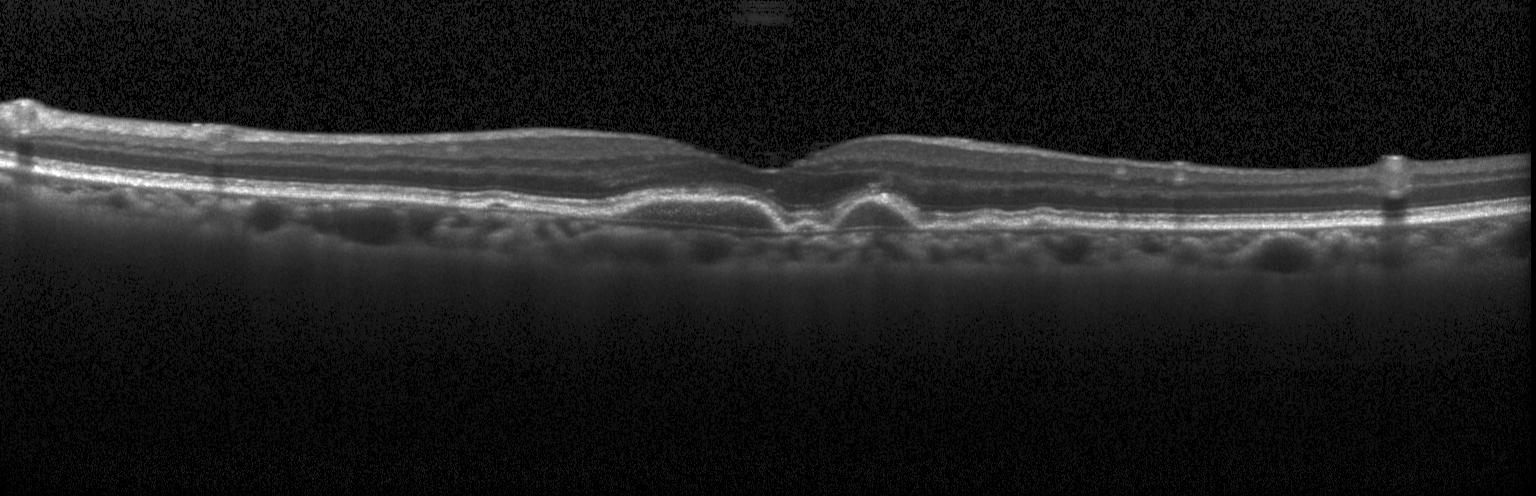

Heidelberg Spectralis · spectral-domain optical coherence tomography · optical coherence tomography B-scan · macular scan.
Diagnosis: CNV.